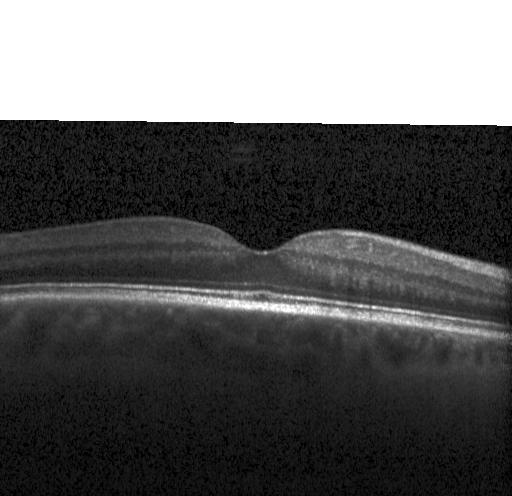 Diagnosis: no evidence of choroidal neovascularization, diabetic macular edema, or drusen.